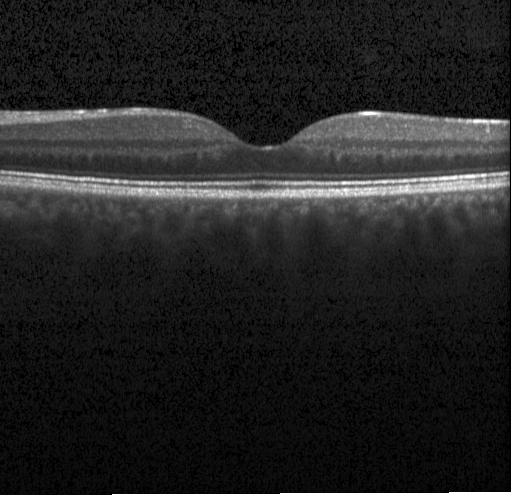

Retinal OCT B-scan. Heidelberg Spectralis. Spectral-domain optical coherence tomography
OCT finding: neither choroidal neovascularization, diabetic macular edema, nor drusen.